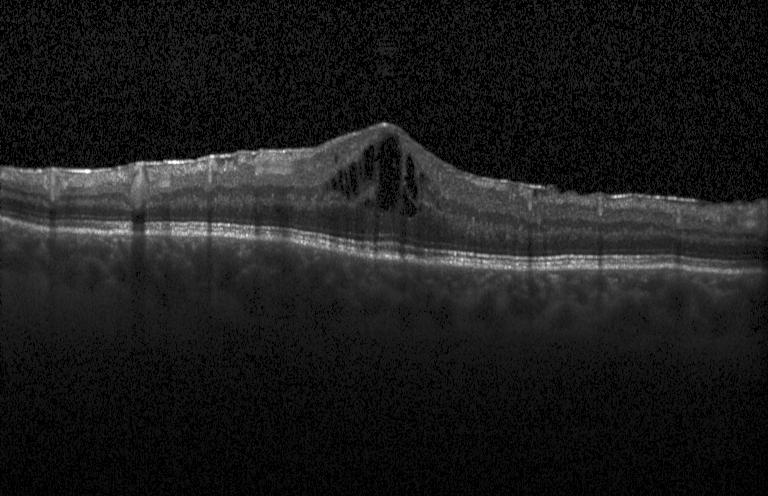

Finding: DME.